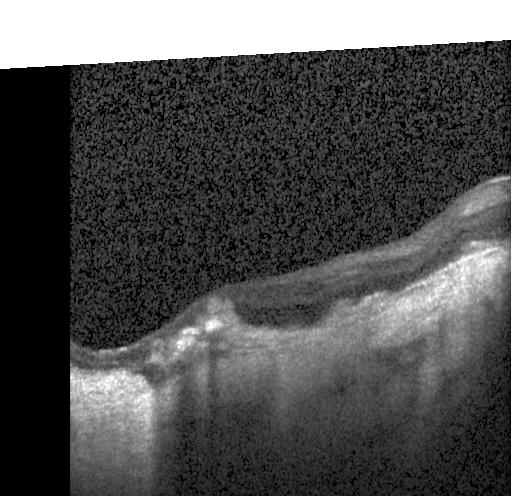 Spectral-domain optical coherence tomography, instrument: Heidelberg Spectralis, optical coherence tomography scan
Impression: choroidal neovascularization (CNV).